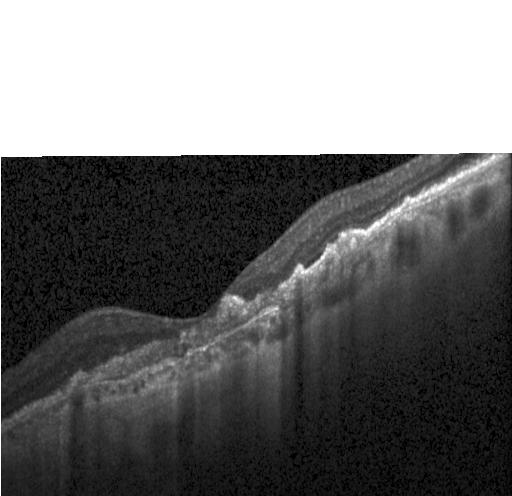

Retinal OCT cross-section showing CNV.